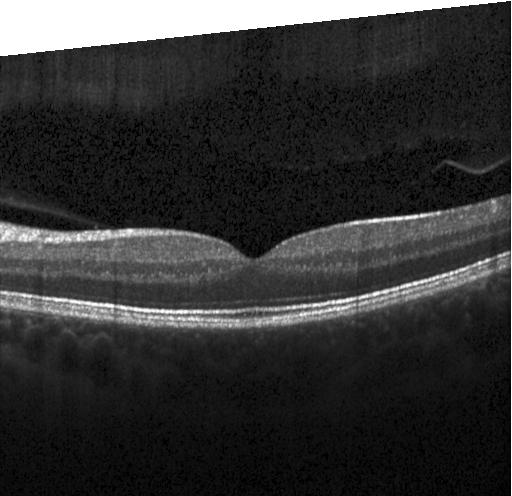

OCT B-scan · acquired on a Heidelberg Spectralis · spectral-domain OCT — Impression: no evidence of CNV, DME, or drusen.